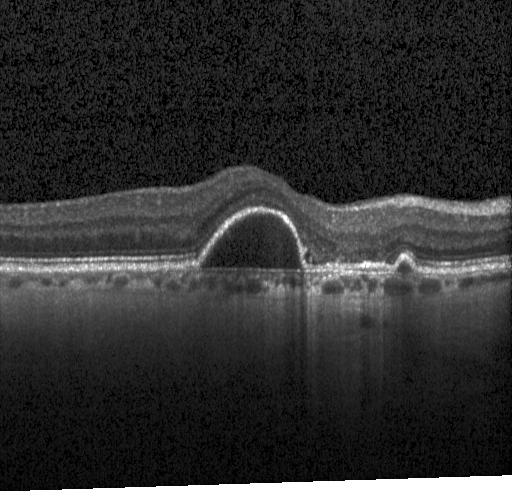 Assessment: choroidal neovascularization.